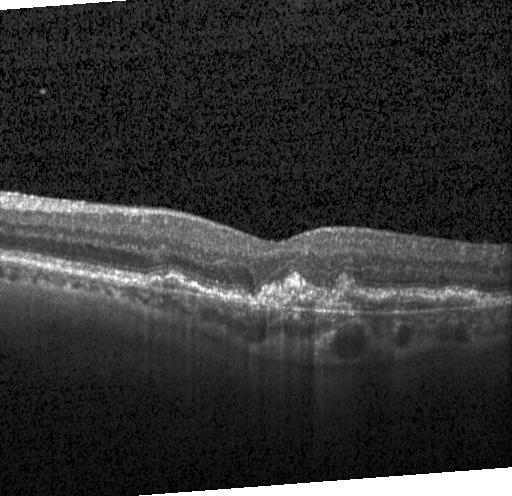

Retinal OCT B-scan — Assessment: choroidal neovascularization (CNV).